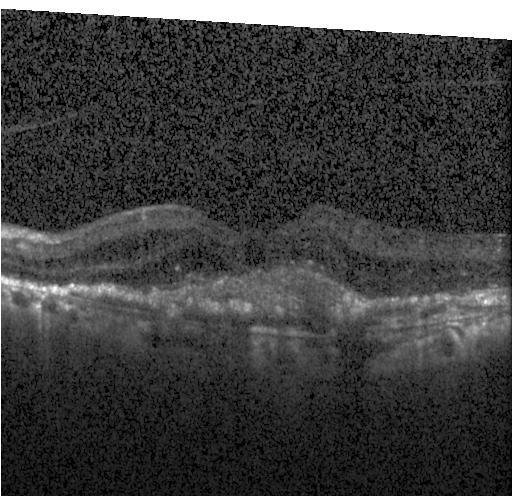 OCT finding: a choroidal neovascular membrane.